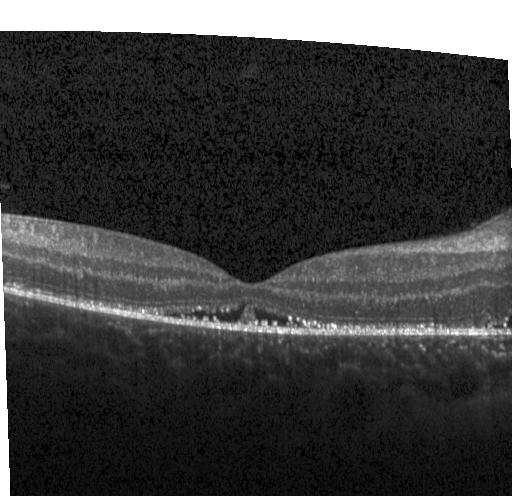 Finding: a choroidal neovascular membrane.